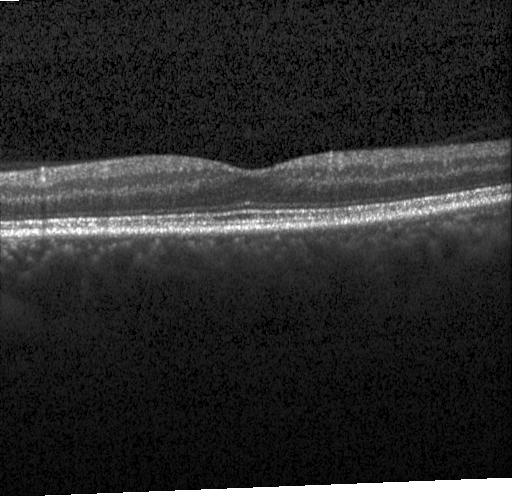

Impression: neither CNV, DME, nor drusen.